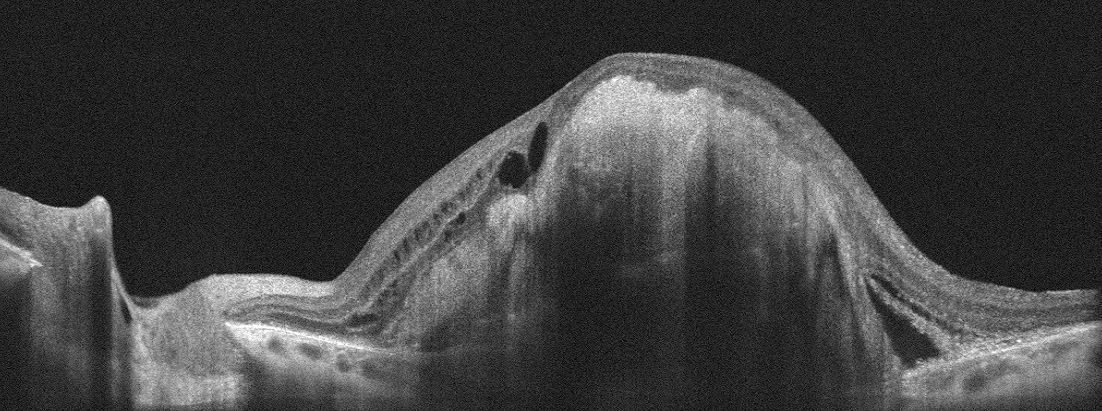

The scan shows AMD.